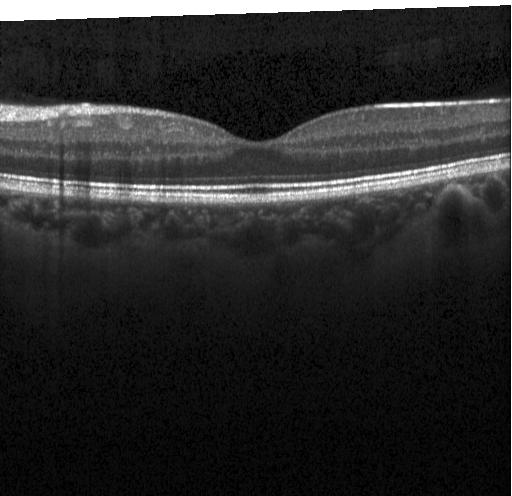
Retinal OCT B-scan. Acquired on a Heidelberg Spectralis. Centered on the fovea. SD-OCT.
Finding: no CNV, DME, or drusen.